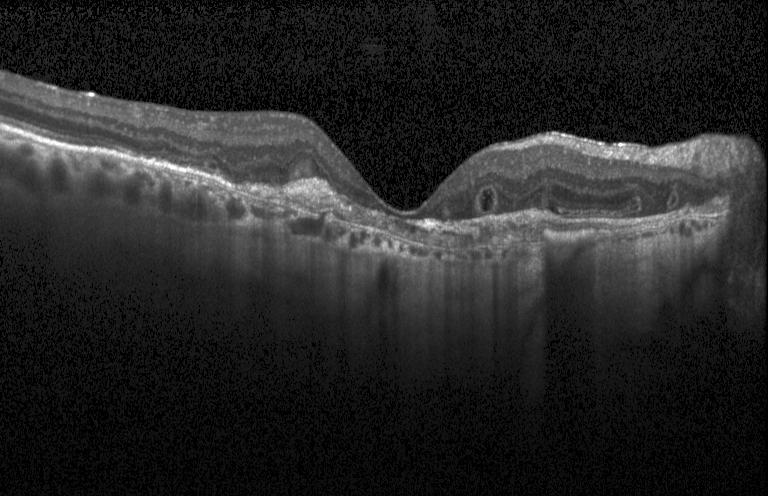

Optical coherence tomography scan, through the macula
Impression: choroidal neovascularization.